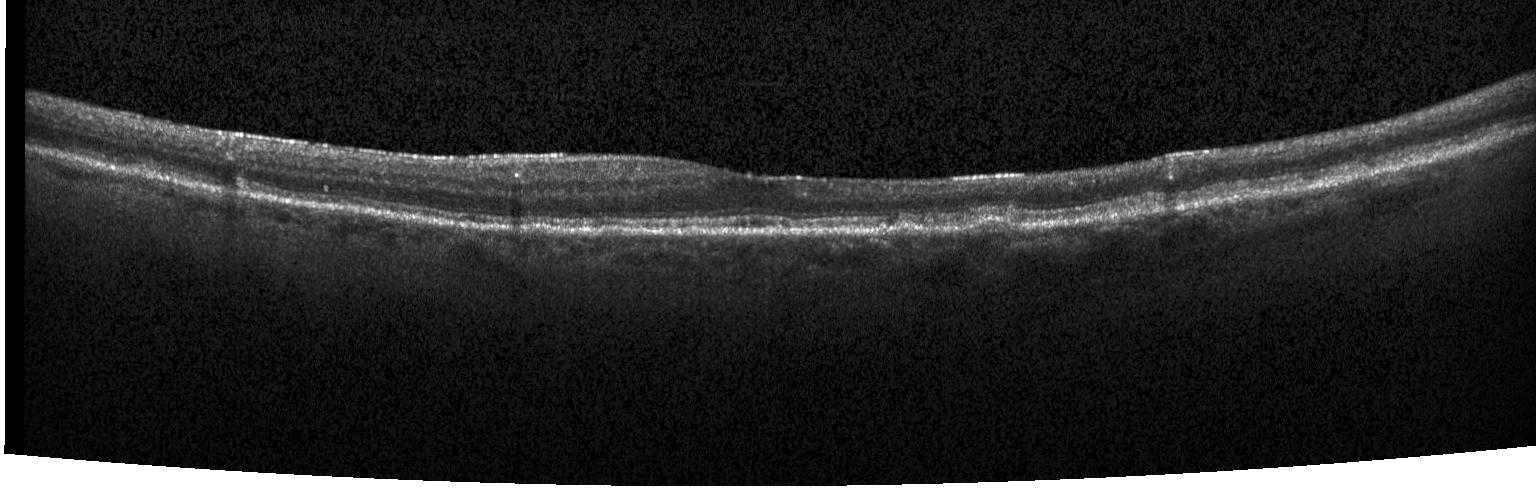
OCT finding: multiple drusen.